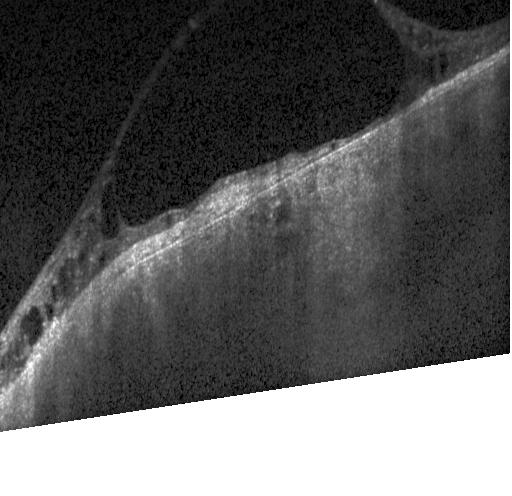 Retinal OCT cross-section · Heidelberg Spectralis — Impression: a choroidal neovascular membrane.